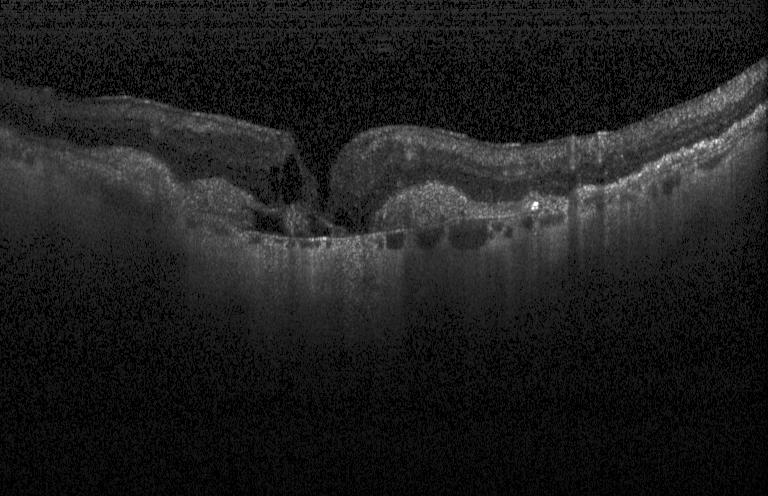

Retinal OCT B-scan; spectral-domain optical coherence tomography.
Dx: choroidal neovascularization.